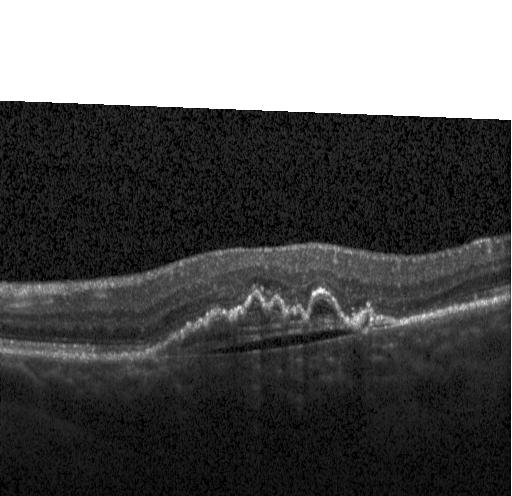 Impression: choroidal neovascularization.